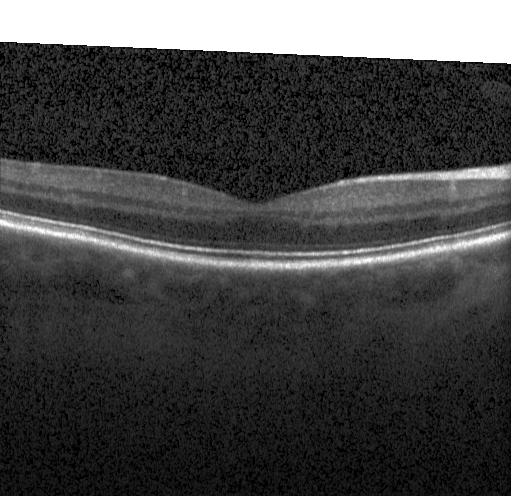

Impression: neither choroidal neovascularization, diabetic macular edema, nor drusen.